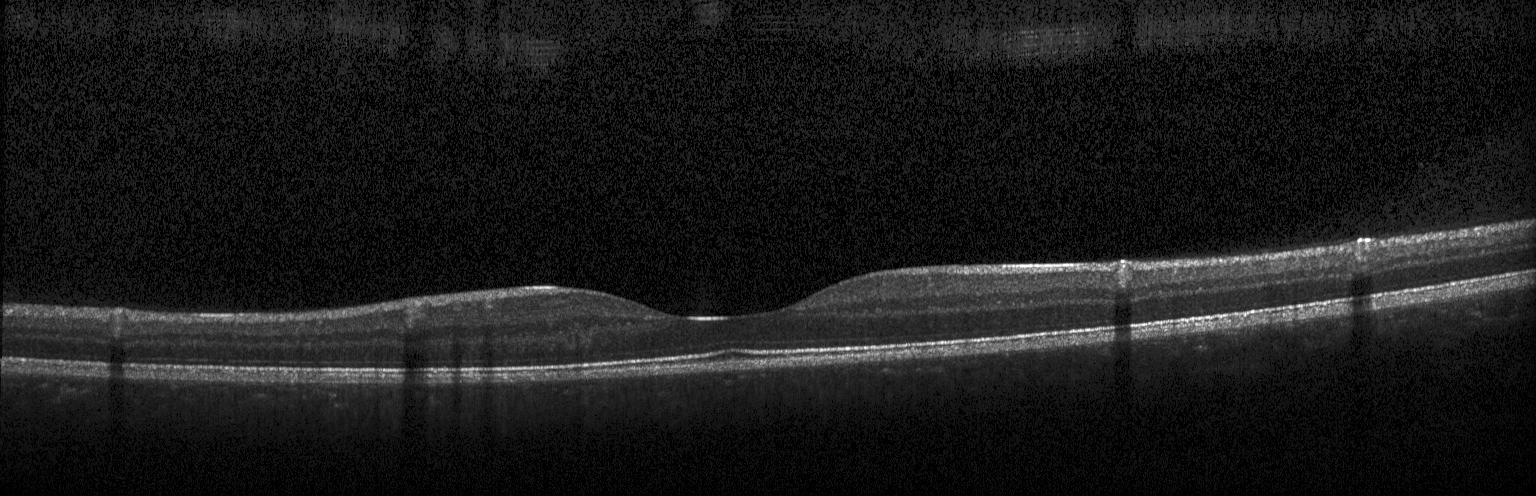 The scan shows neither choroidal neovascularization, diabetic macular edema, nor drusen.